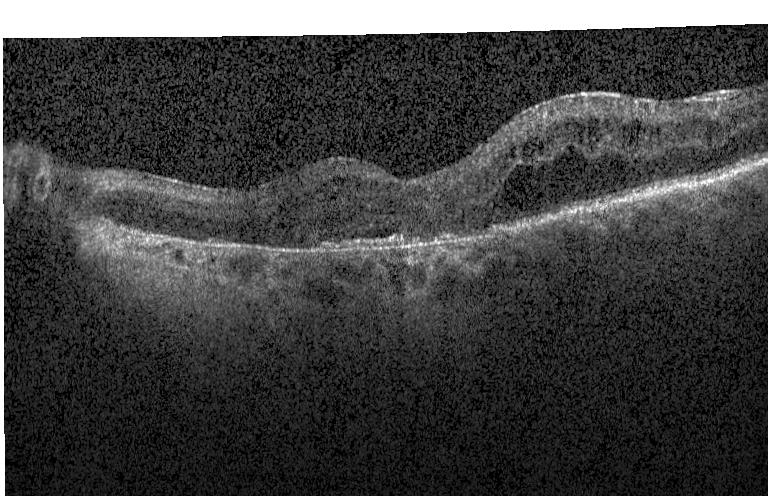
Heidelberg Spectralis OCT system. Retinal OCT B-scan. Horizontal scan through the fovea. Spectral-domain optical coherence tomography
Impression: a choroidal neovascular membrane.